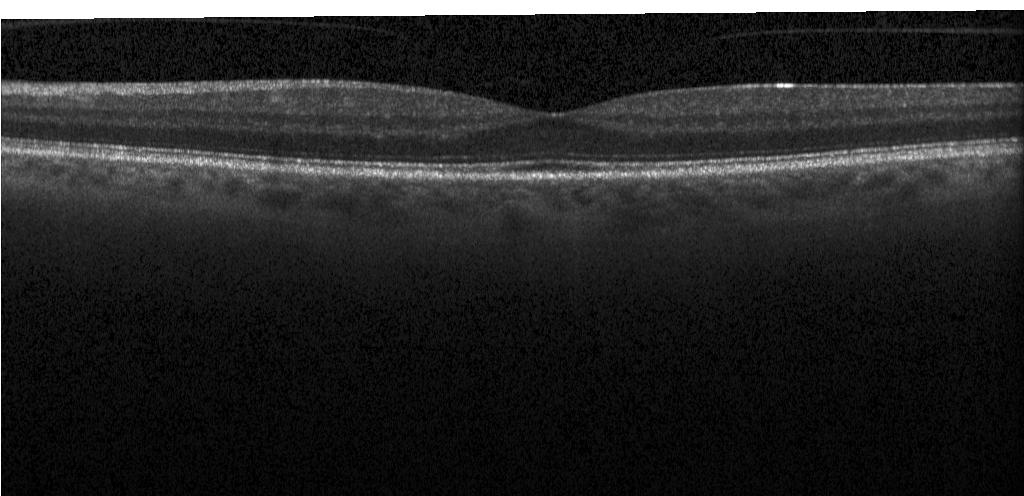
Retinal OCT cross-section · Heidelberg Spectralis. Impression: no CNV, DME, or drusen.